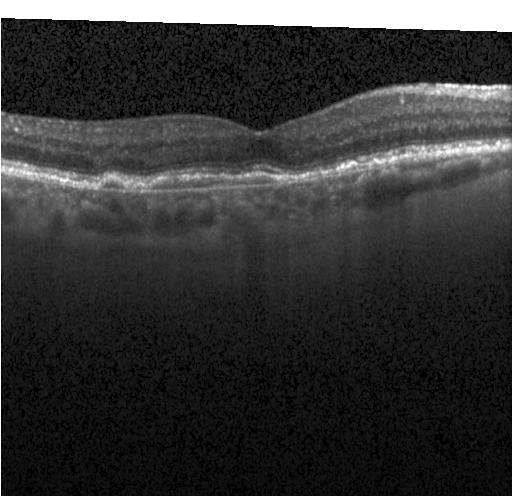

Impression: a choroidal neovascular membrane.